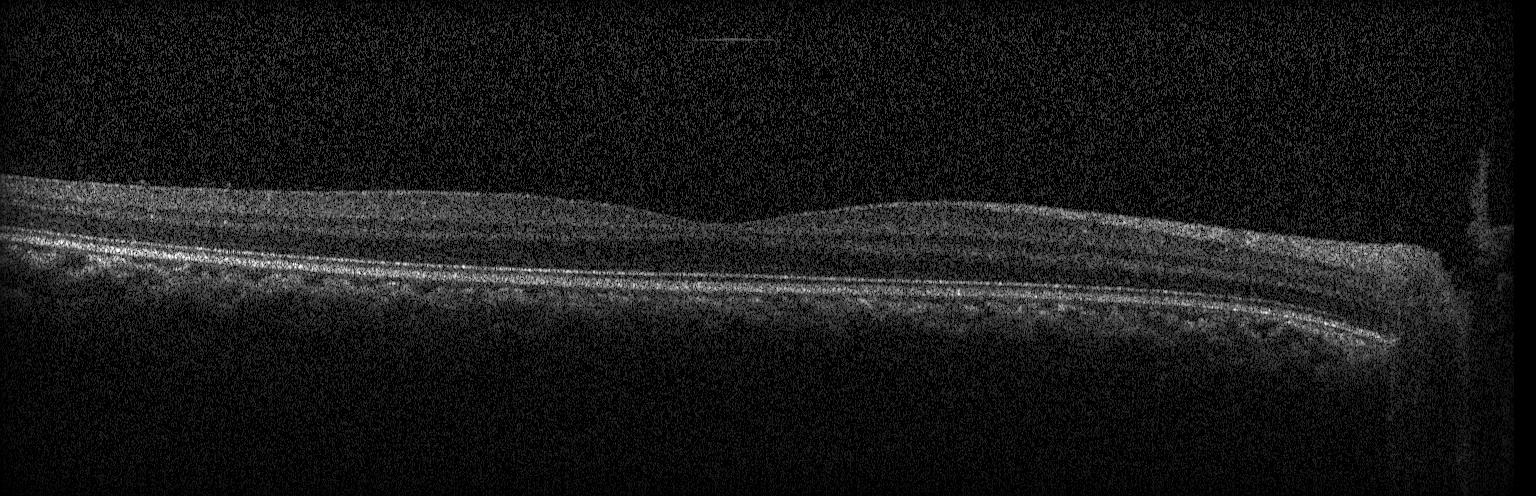
Retinal OCT B-scan · fovea-centered · Heidelberg Spectralis OCT system · spectral-domain optical coherence tomography — The scan shows no CNV, no DME, and no drusen.